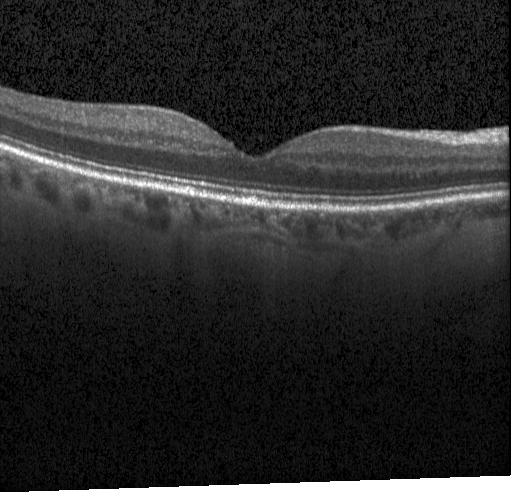 Retinal OCT cross-section showing no choroidal neovascularization, diabetic macular edema, or drusen.